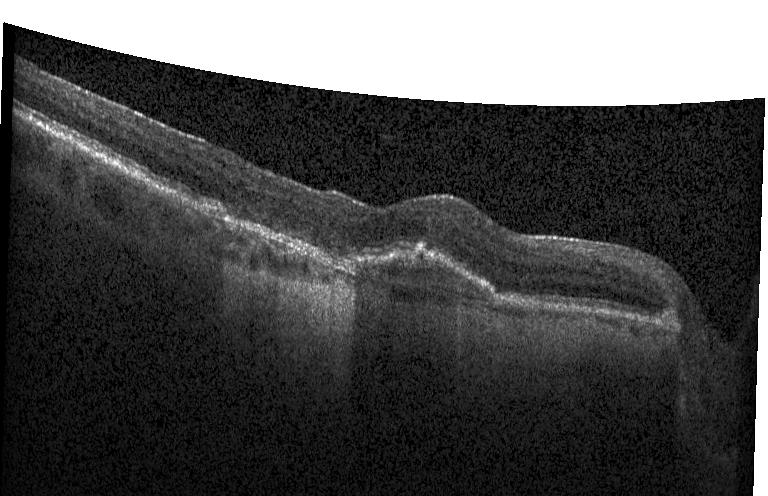

Finding: CNV.